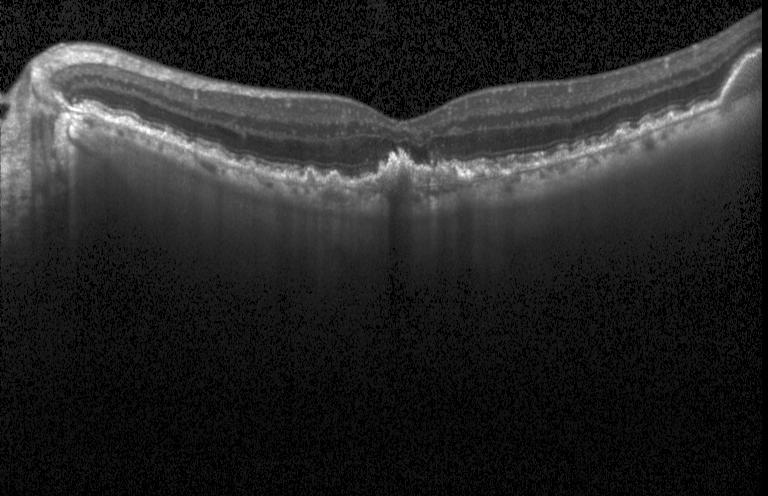 OCT line scan
Diagnosis: a choroidal neovascular membrane.